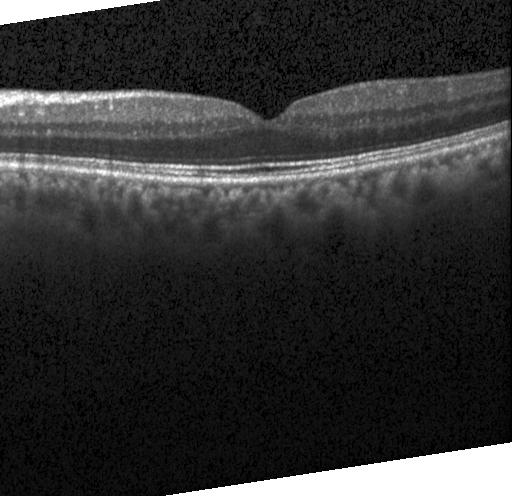
Spectral-domain OCT. Acquired on a Heidelberg Spectralis. OCT line scan. Through the macula
Impression: no choroidal neovascularization, diabetic macular edema, or drusen.